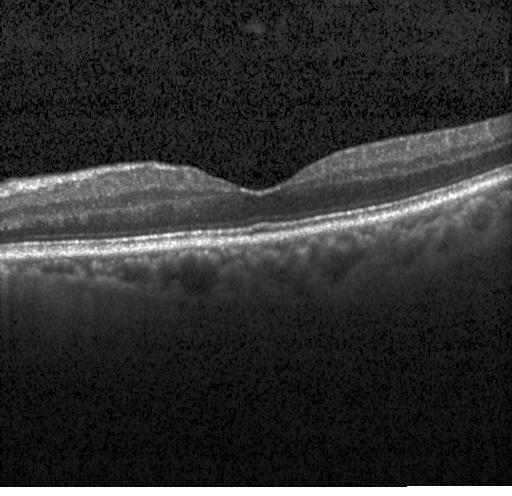 This B-scan demonstrates no evidence of CNV, DME, or drusen.